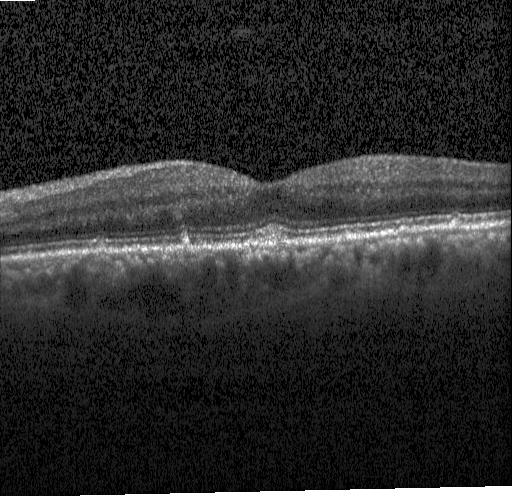
This B-scan demonstrates drusen.